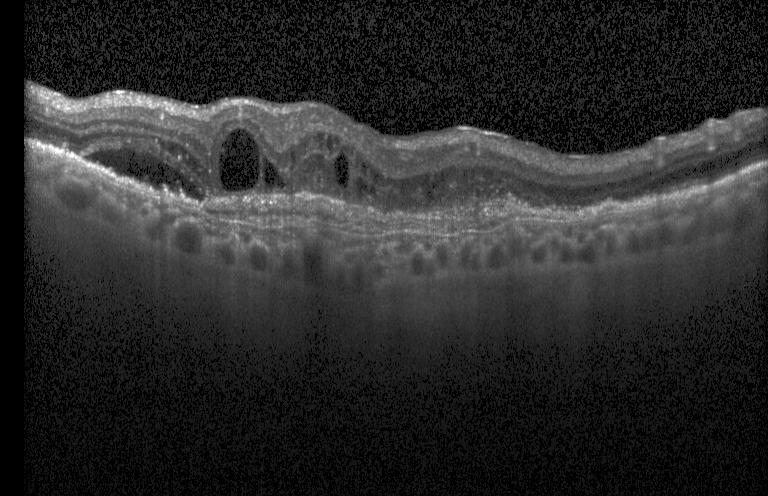
Dx: a choroidal neovascular membrane.